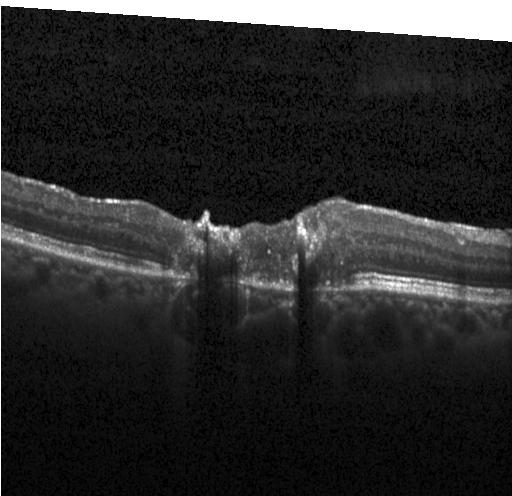 OCT B-scan. Diagnosis: a choroidal neovascular membrane.